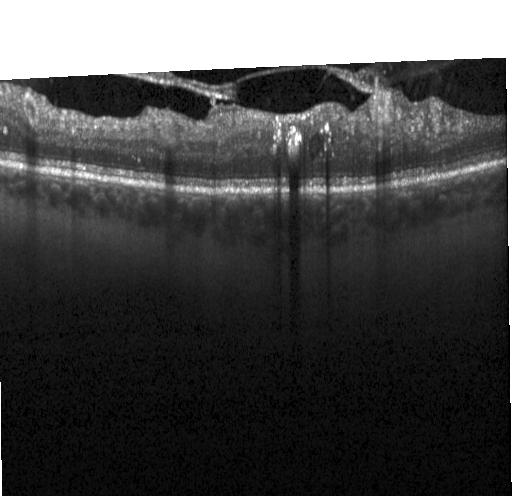
Dx: DME.